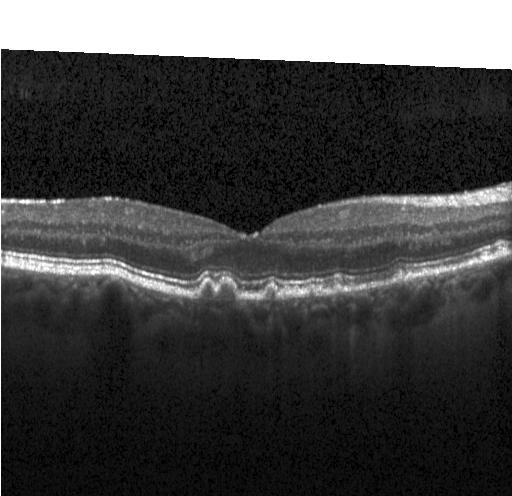 OCT line scan. Dx: sub-RPE drusenoid deposits.